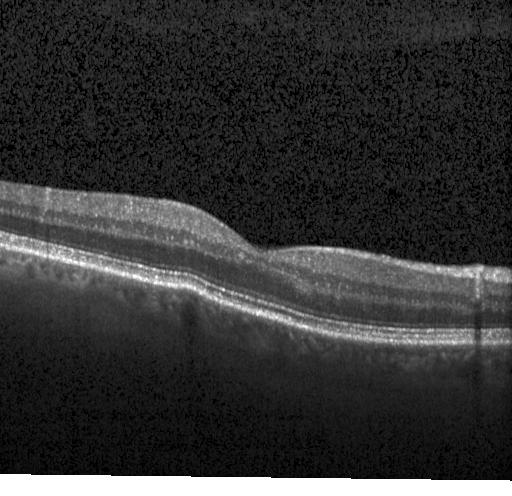
OCT B-scan — Dx: no evidence of choroidal neovascularization, diabetic macular edema, or drusen.